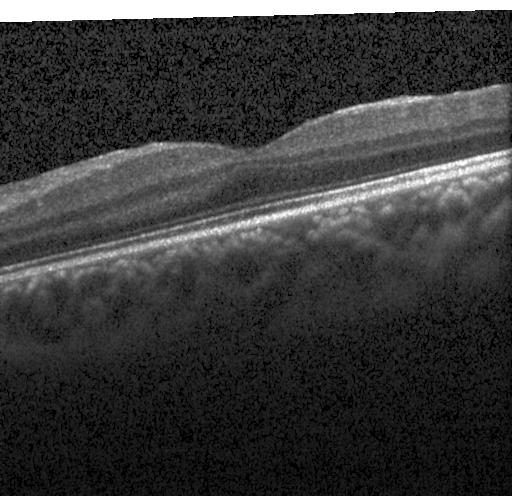

This B-scan demonstrates no CNV, no DME, and no drusen.